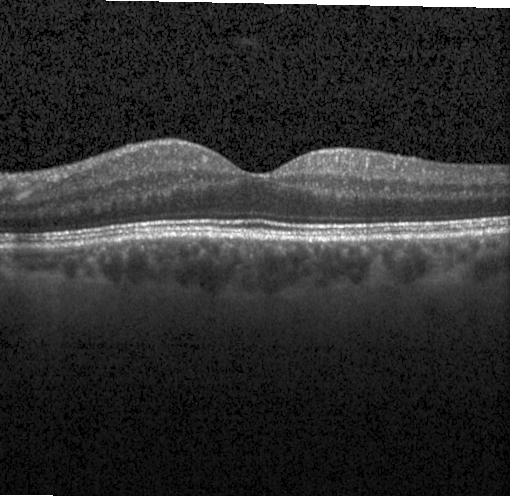

Spectral-domain OCT B-scan: no choroidal neovascularization, diabetic macular edema, or drusen.